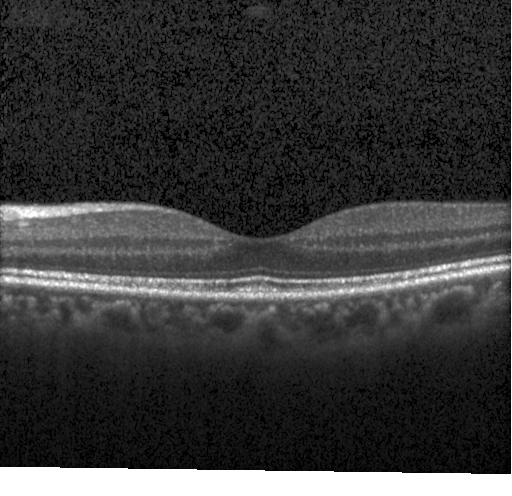
Optical coherence tomography B-scan.
Diagnosis: no evidence of CNV, DME, or drusen.